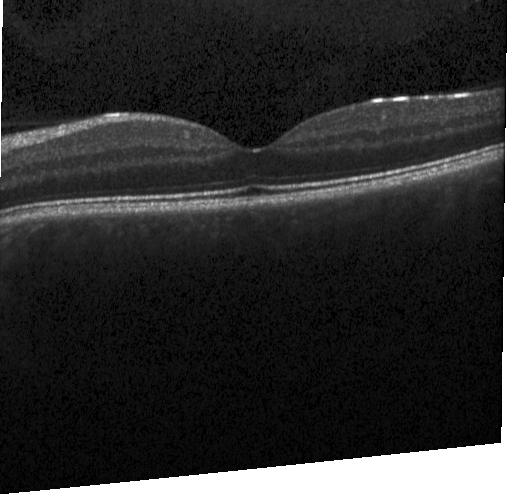 OCT finding: no choroidal neovascularization, no diabetic macular edema, and no drusen.